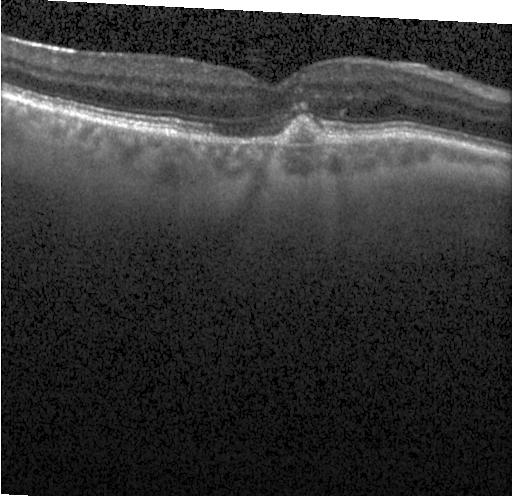
Optical coherence tomography B-scan; SD-OCT — This B-scan demonstrates a choroidal neovascular membrane.